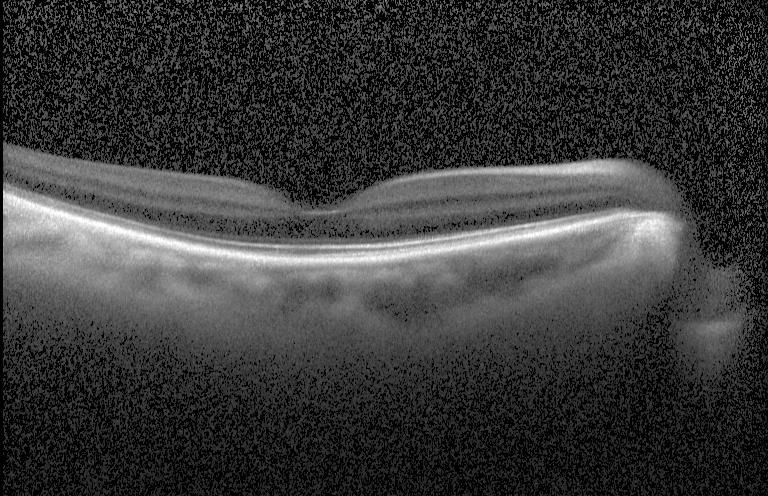
Heidelberg Spectralis. OCT line scan.
Assessment: no evidence of CNV, DME, or drusen.